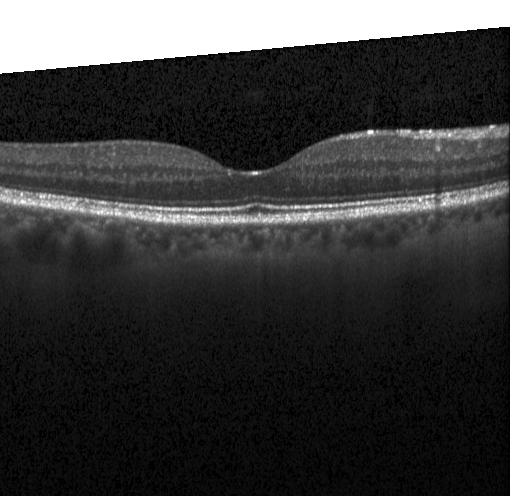

Instrument: Heidelberg Spectralis; SD-OCT; retinal OCT B-scan.
Dx: neither choroidal neovascularization, diabetic macular edema, nor drusen.